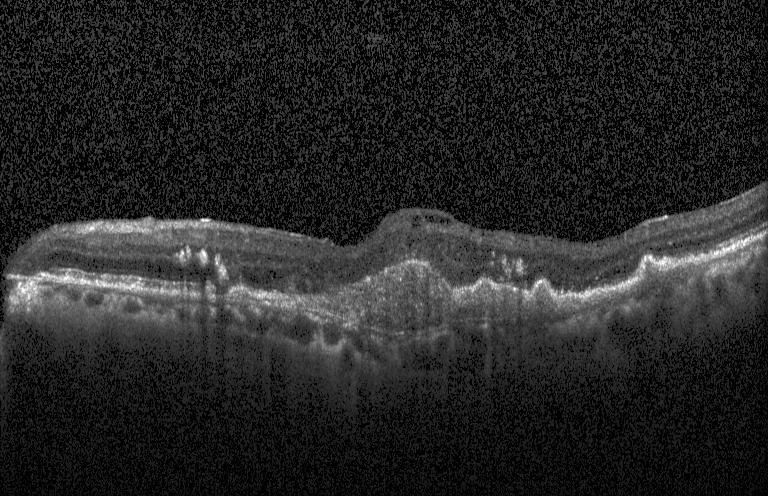
Spectral-domain optical coherence tomography. Instrument: Heidelberg Spectralis. OCT B-scan — Finding: a choroidal neovascular membrane.